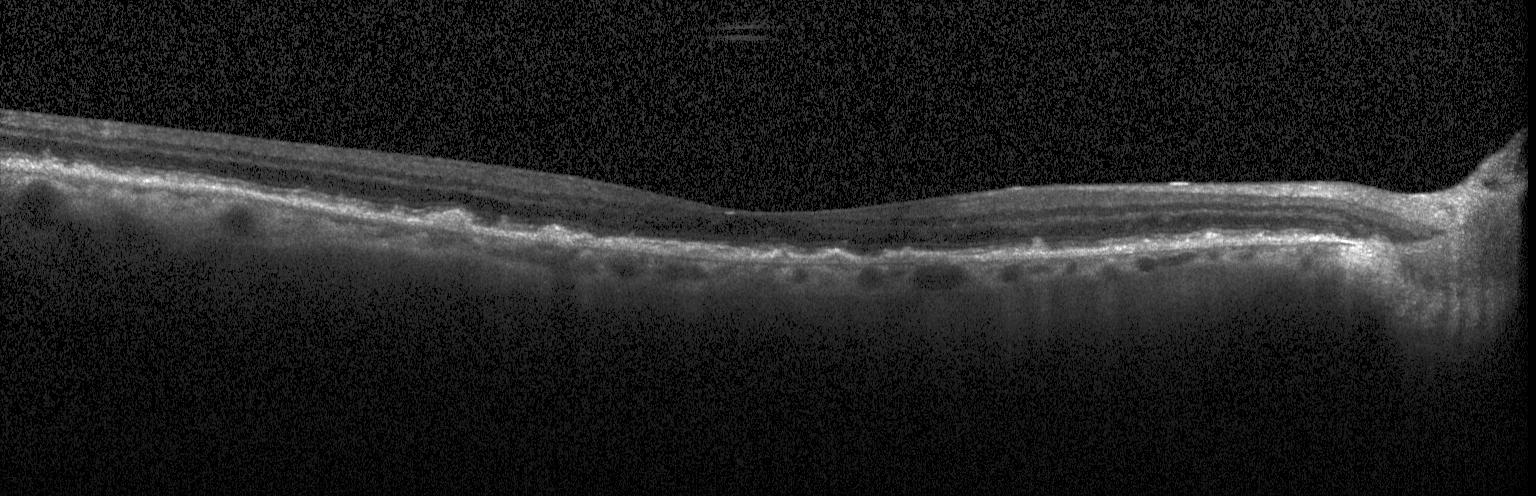 Horizontal scan through the fovea. OCT B-scan. Instrument: Heidelberg Spectralis. Spectral-domain optical coherence tomography. Impression: choroidal neovascularization (CNV).